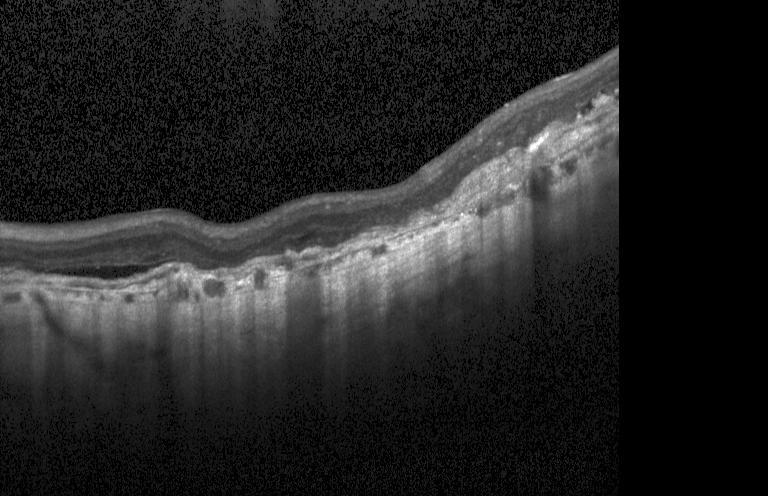

Spectral-domain optical coherence tomography; retinal OCT cross-section; Heidelberg Spectralis; macular scan.
Finding: a choroidal neovascular membrane.